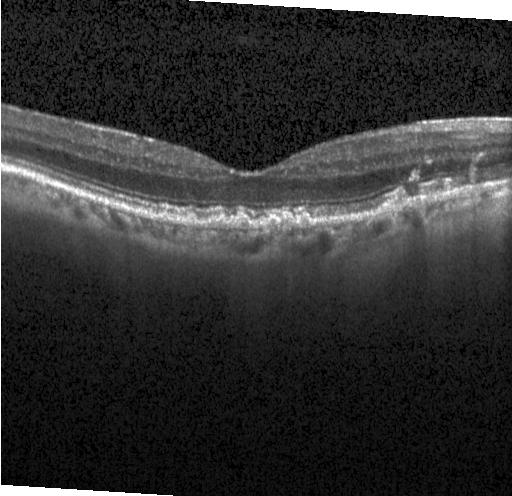 OCT B-scan. Macular OCT: multiple drusen.